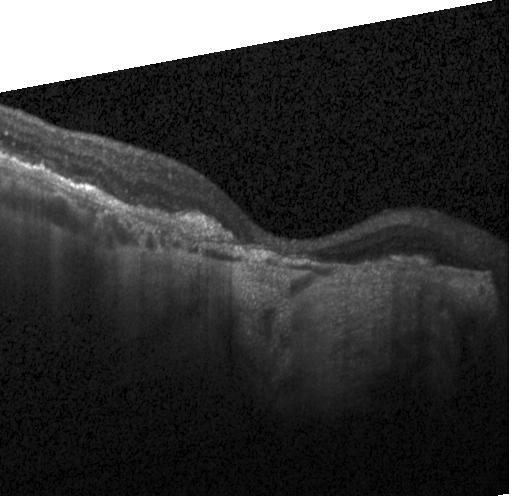 Diagnosis: a choroidal neovascular membrane.